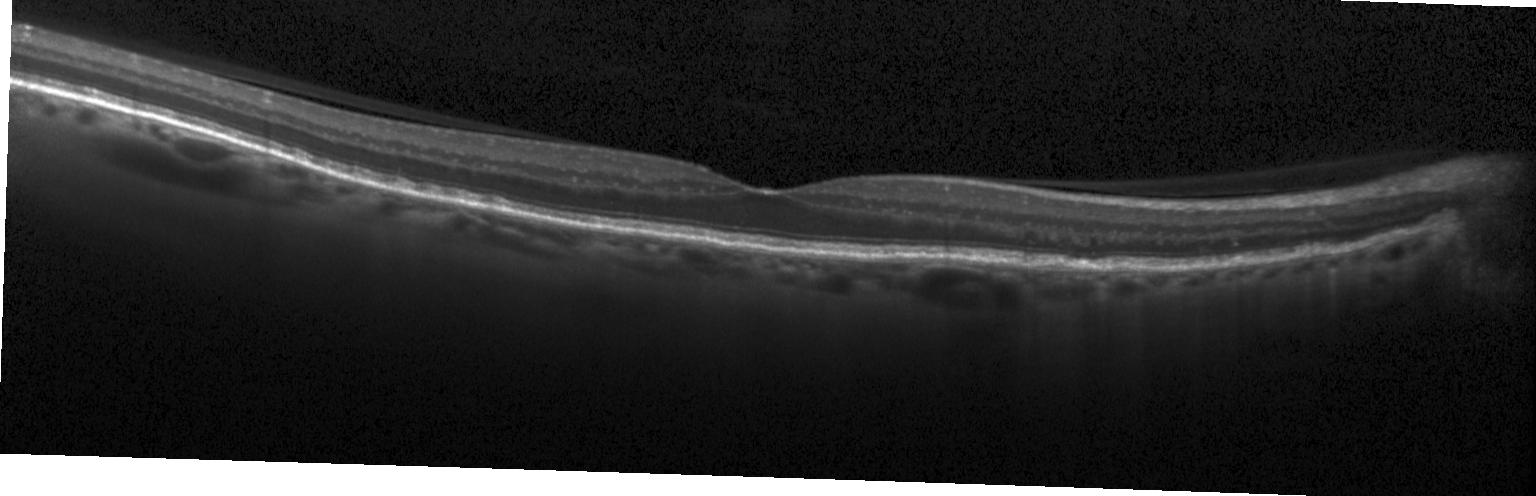
Retinal OCT cross-section.
The scan shows no choroidal neovascularization, no diabetic macular edema, and no drusen.